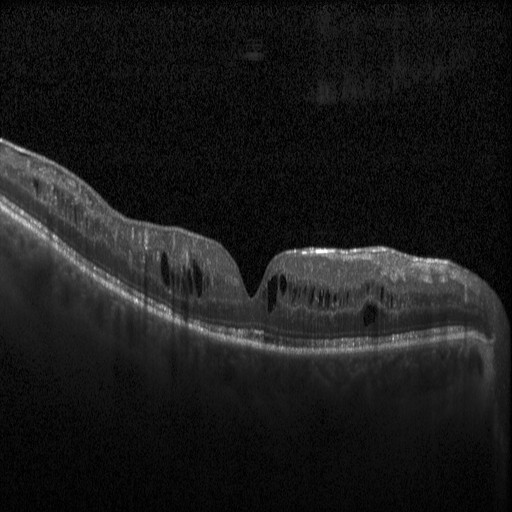
Through the macula, instrument: Heidelberg Spectralis, SD-OCT, OCT B-scan. Diagnosis: diabetic macular edema (DME).